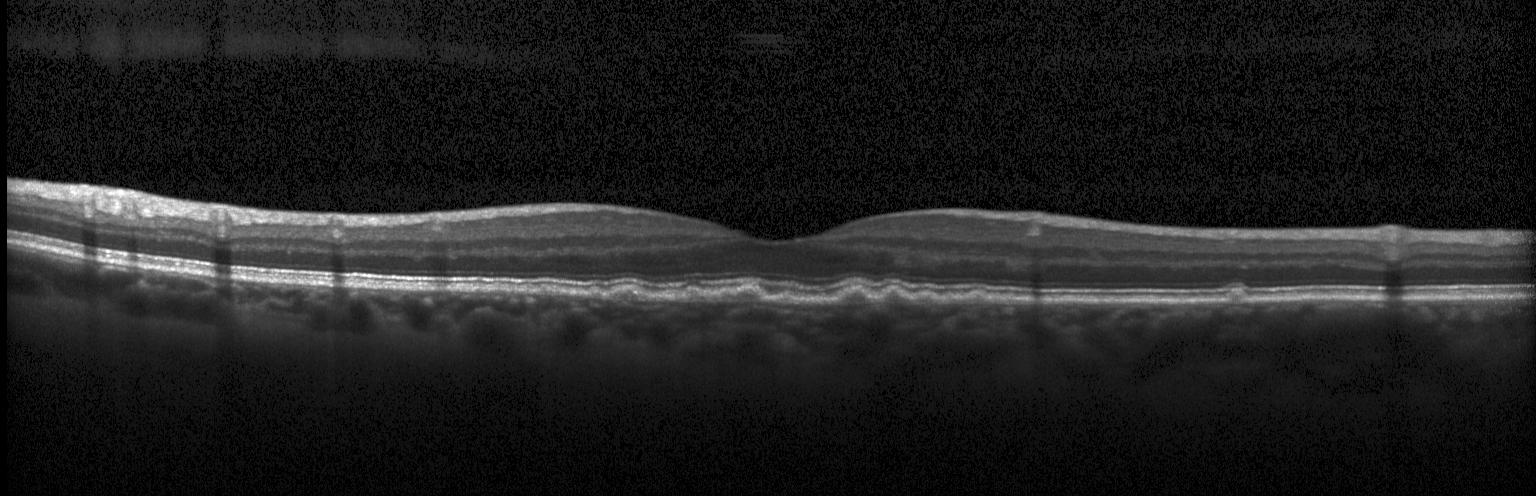
Retinal OCT B-scan — Finding: sub-RPE drusenoid deposits.